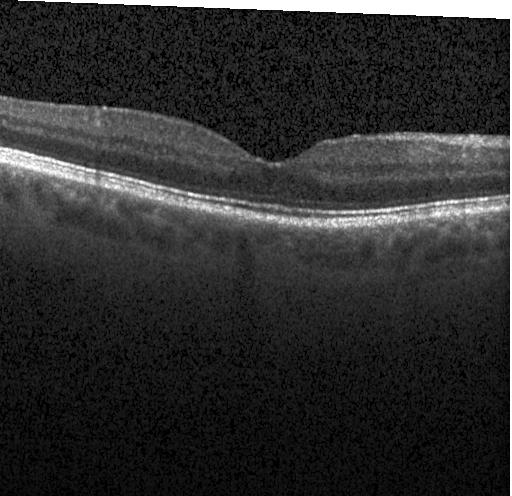 Optical coherence tomography B-scan; Heidelberg Spectralis. This B-scan demonstrates no evidence of choroidal neovascularization, diabetic macular edema, or drusen.